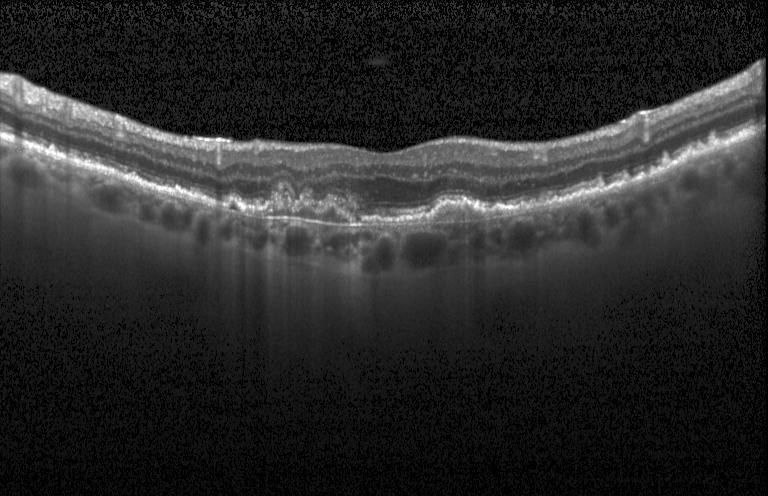

Retinal OCT cross-section, through the macula, instrument: Heidelberg Spectralis.
OCT finding: a choroidal neovascular membrane.